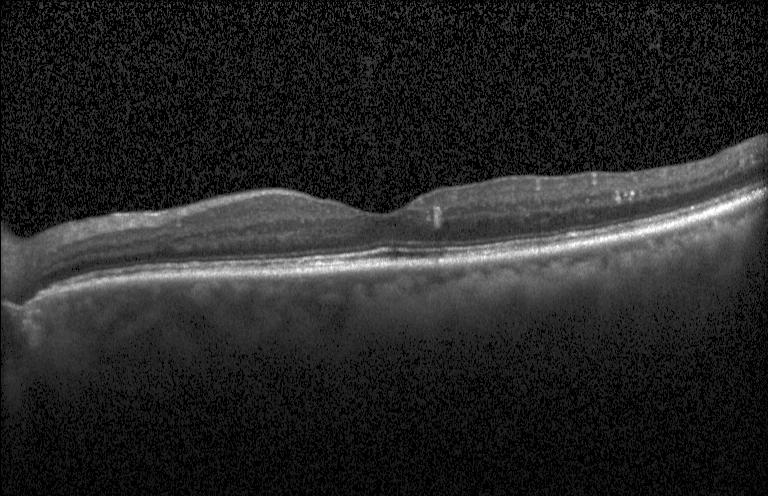

Finding: no evidence of choroidal neovascularization, diabetic macular edema, or drusen.